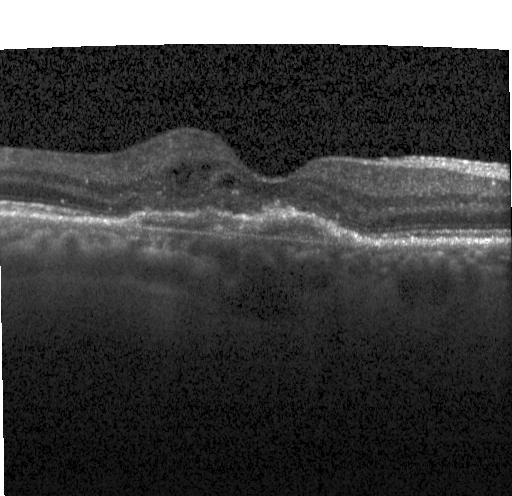
OCT B-scan
A choroidal neovascular membrane.